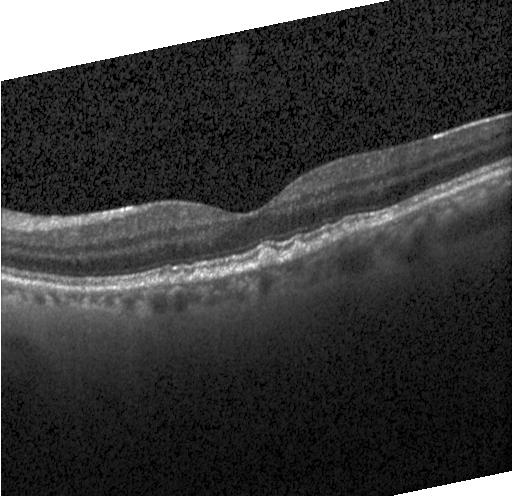
Retinal OCT cross-section — Diagnosis: drusen.